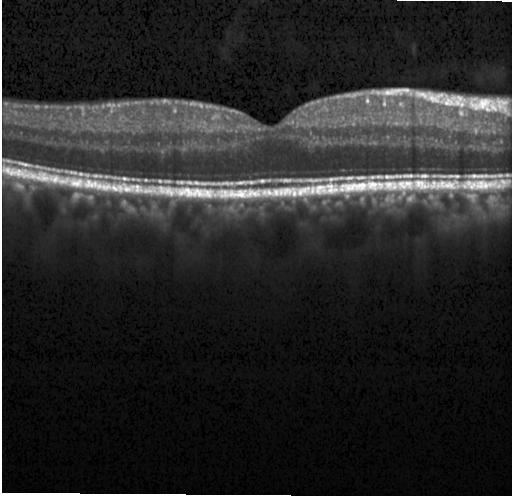
Acquired on a Heidelberg Spectralis. Optical coherence tomography scan
OCT finding: no choroidal neovascularization, diabetic macular edema, or drusen.